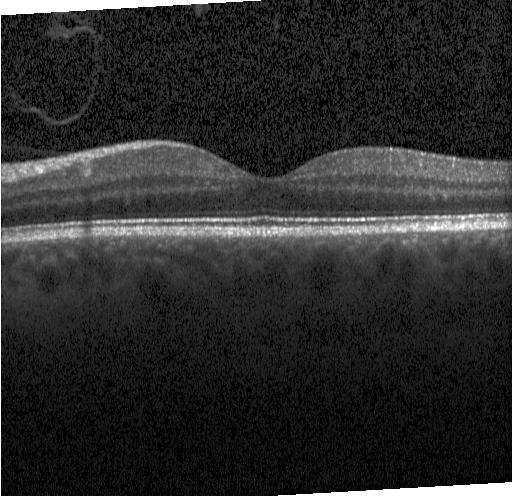 SD-OCT. Through the macula. OCT line scan — The scan shows no choroidal neovascularization, no diabetic macular edema, and no drusen.